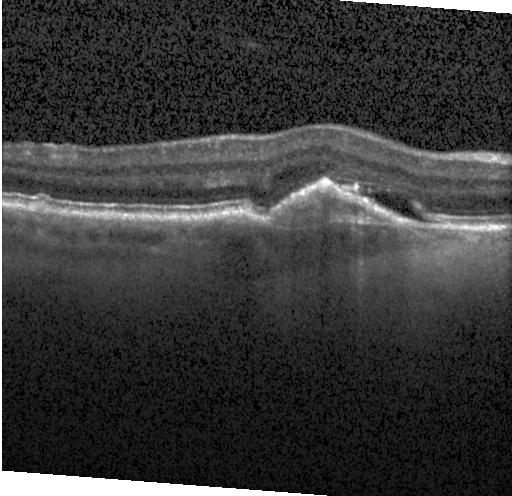 Optical coherence tomography scan. SD-OCT.
OCT finding: a choroidal neovascular membrane.